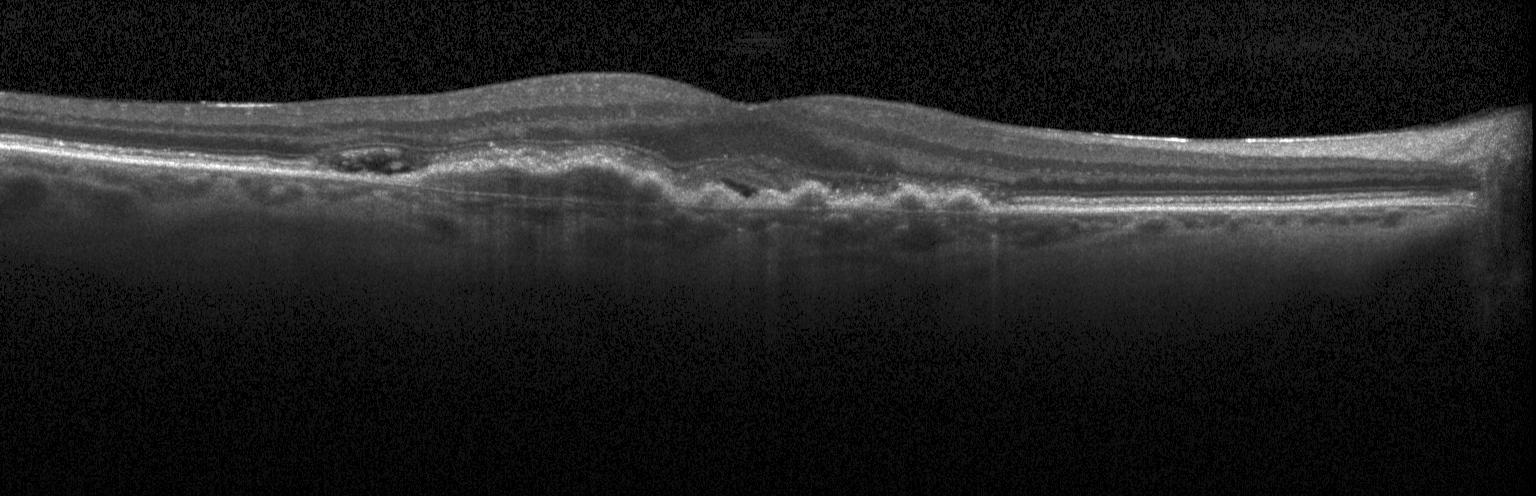 Retinal OCT cross-section
This B-scan demonstrates a choroidal neovascular membrane.